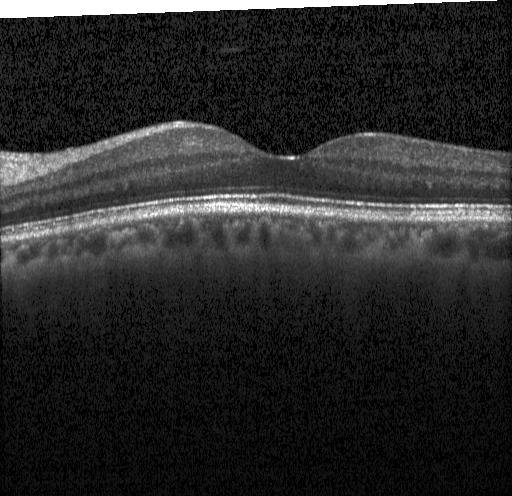
OCT finding: no evidence of CNV, DME, or drusen.